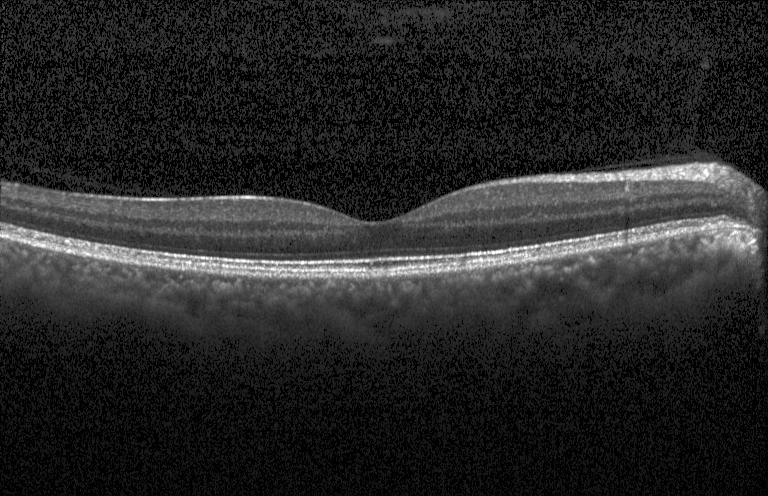 Diagnosis: neither choroidal neovascularization, diabetic macular edema, nor drusen.